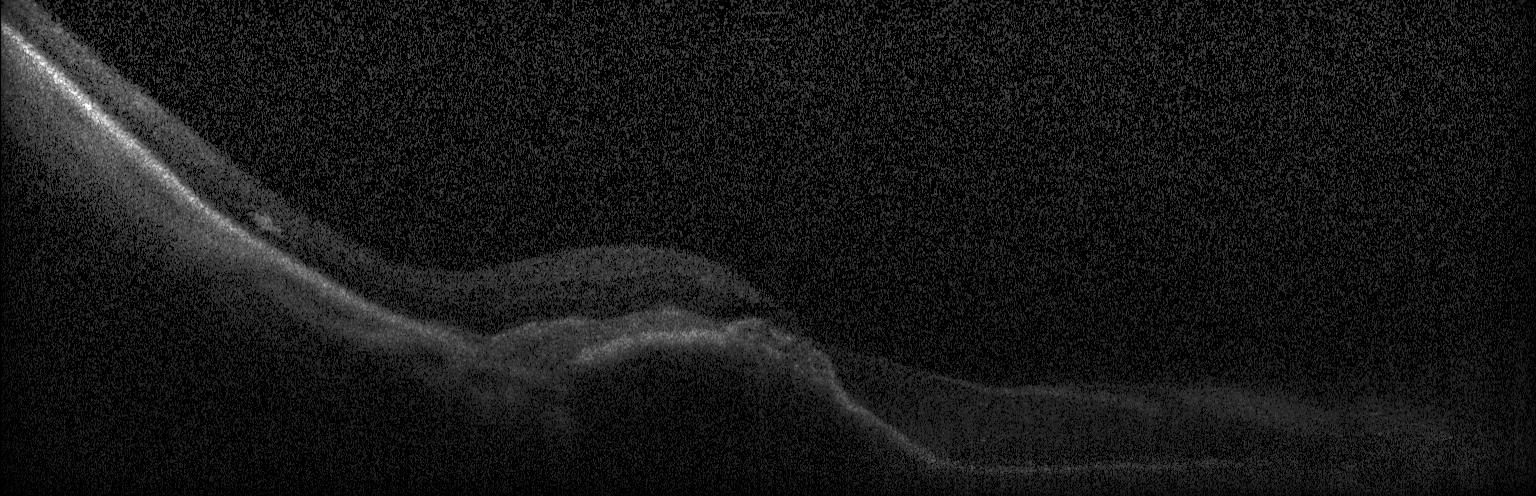

Spectral-domain OCT B-scan: choroidal neovascularization (CNV).